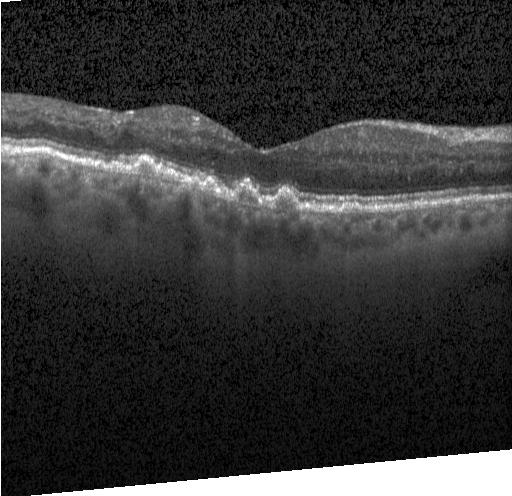 Sub-RPE drusenoid deposits.